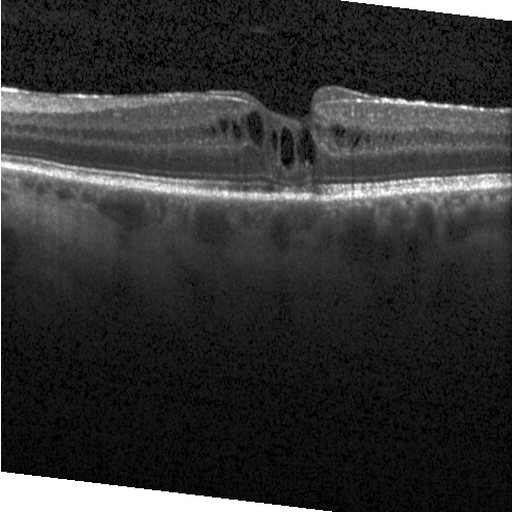
The scan shows DME.